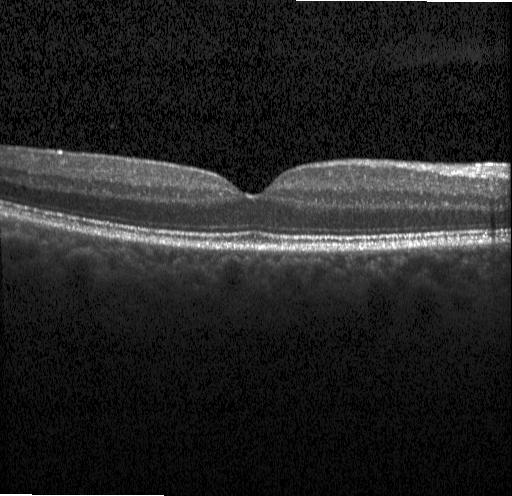
Retinal OCT B-scan — No choroidal neovascularization, no diabetic macular edema, and no drusen.